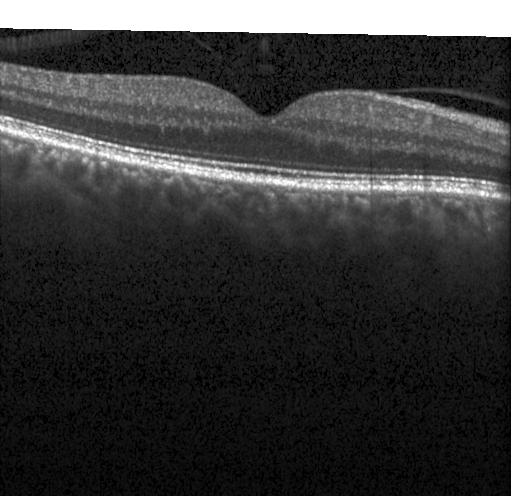
Horizontal scan through the fovea. Retinal OCT B-scan.
The scan shows neither choroidal neovascularization, diabetic macular edema, nor drusen.